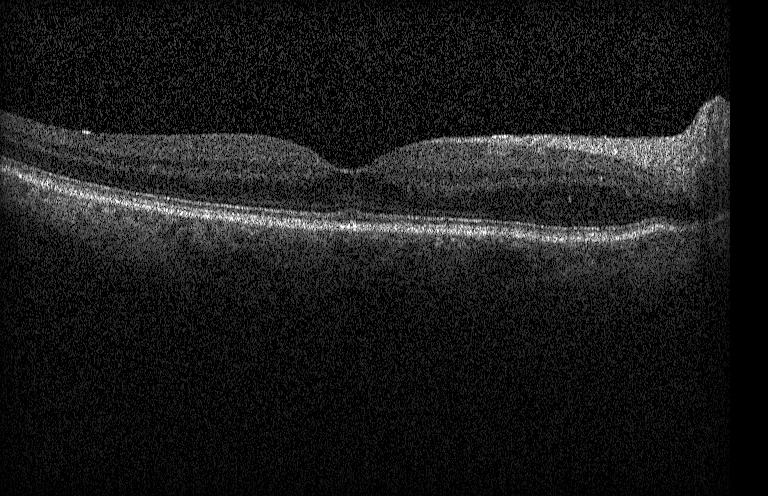

Diagnosis: neither choroidal neovascularization, diabetic macular edema, nor drusen.